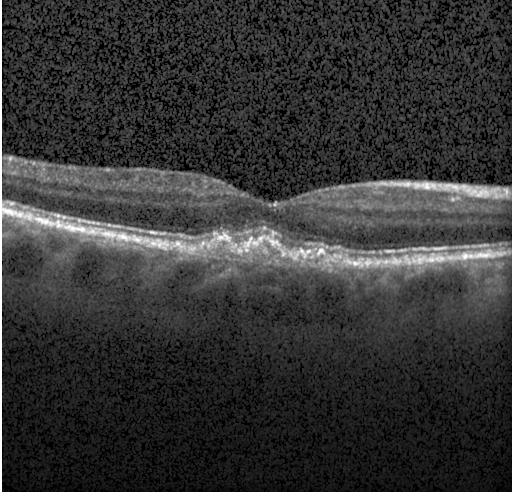
Heidelberg Spectralis, optical coherence tomography scan, SD-OCT — The scan shows sub-RPE drusenoid deposits.